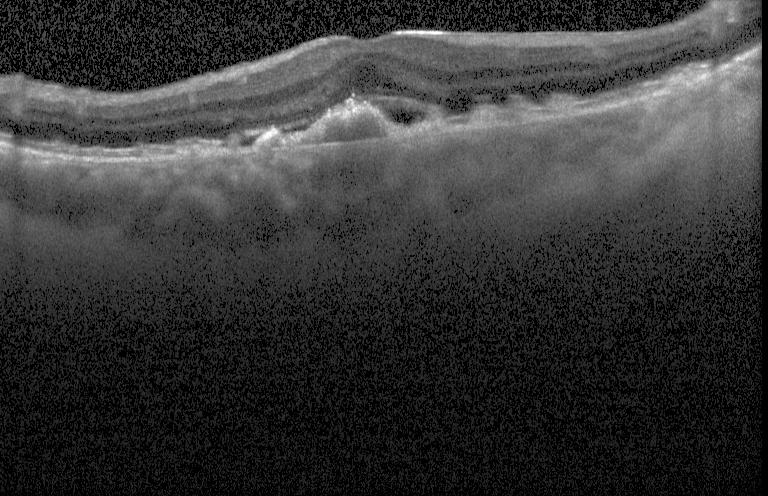
OCT B-scan
Macular OCT: CNV.